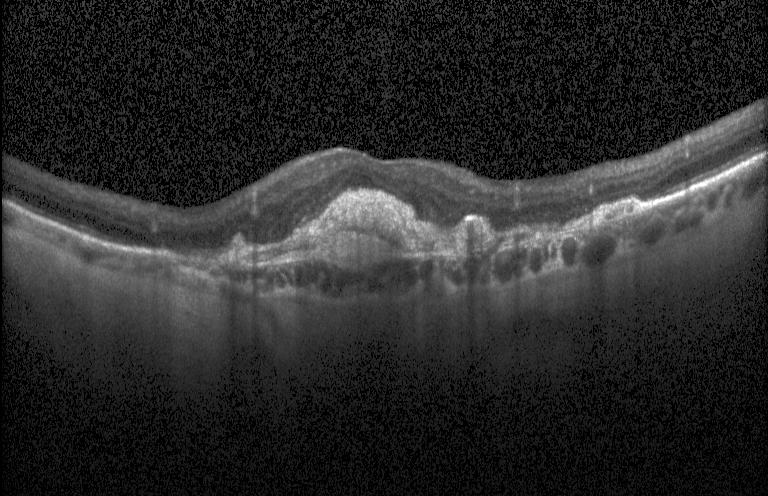

Macular scan, Heidelberg Spectralis, OCT line scan.
A choroidal neovascular membrane.